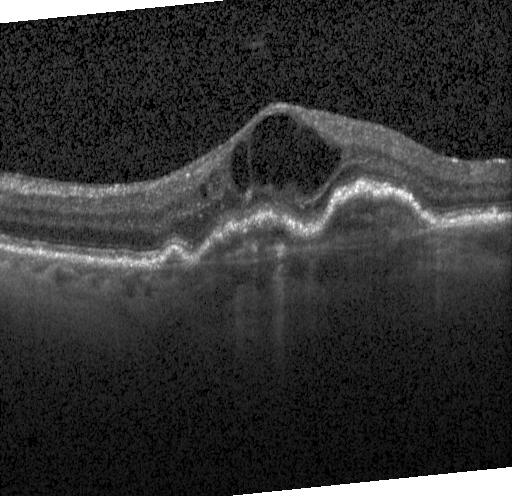
Optical coherence tomography scan, fovea-centered. Choroidal neovascularization (CNV).